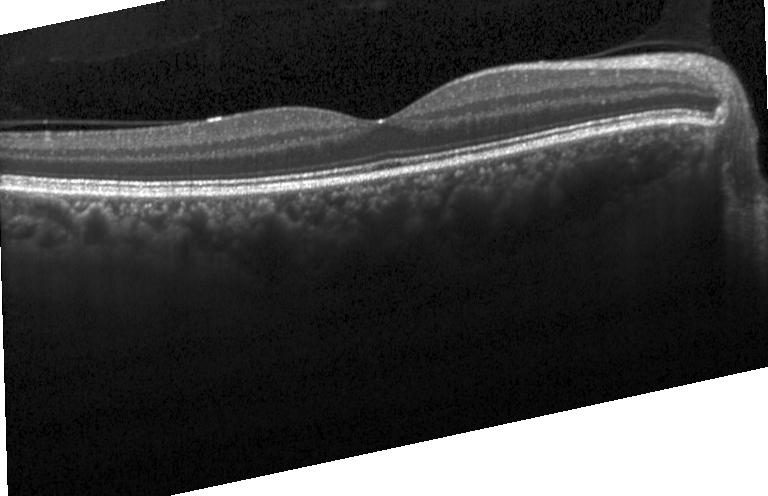 Spectral-domain optical coherence tomography, retinal OCT B-scan, centered on the fovea. Dx: neither CNV, DME, nor drusen.